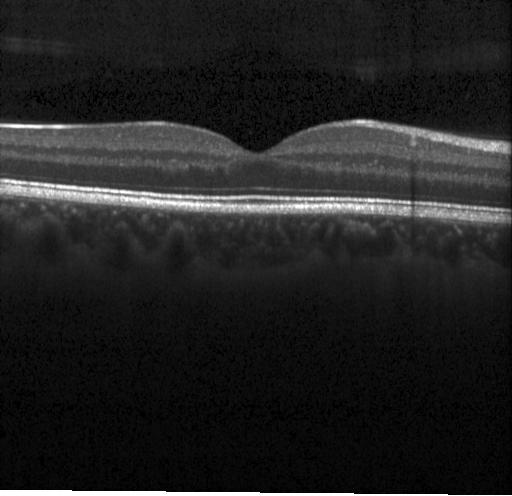
Macular OCT demonstrating no choroidal neovascularization, diabetic macular edema, or drusen.